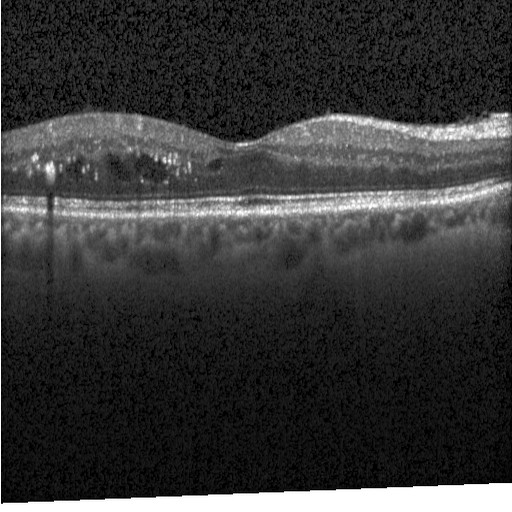

The scan shows DME.